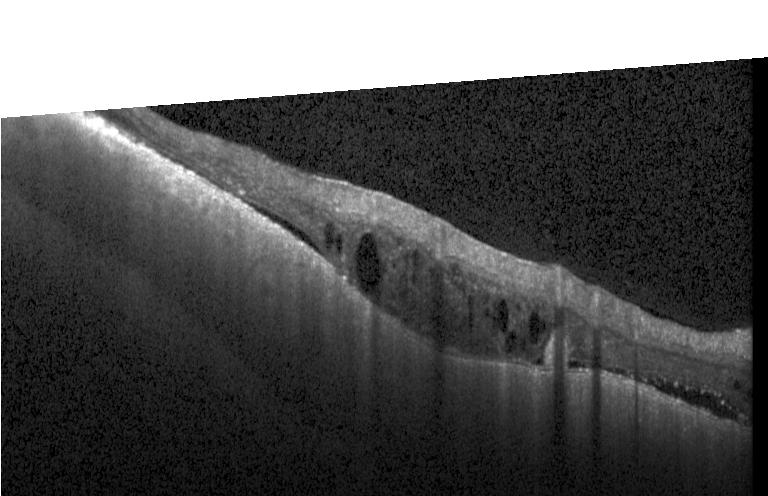
Heidelberg Spectralis OCT system. OCT B-scan. Spectral-domain OCT. Assessment: a choroidal neovascular membrane.